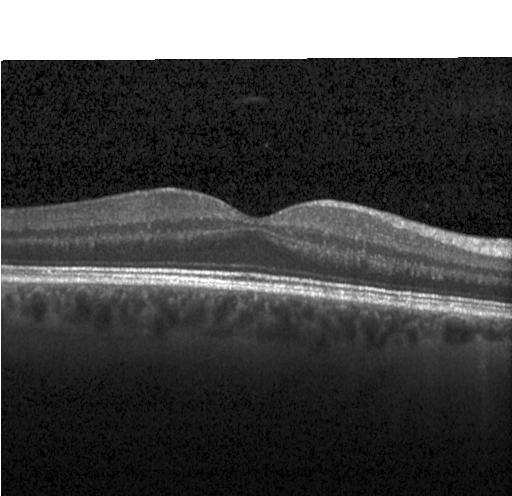
Spectral-domain OCT; OCT line scan; Heidelberg Spectralis. Assessment: no CNV, no DME, and no drusen.